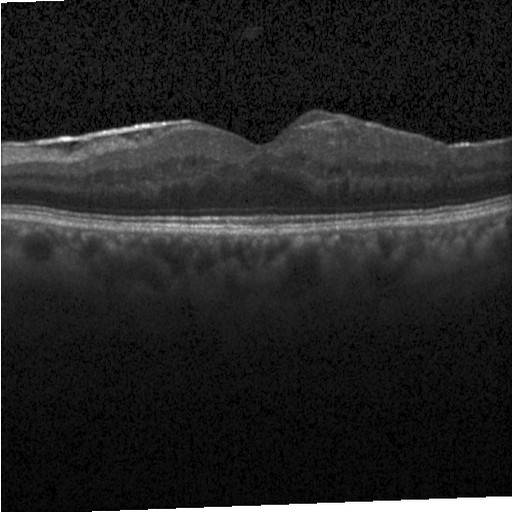

Diagnosis: diabetic macular edema (DME).